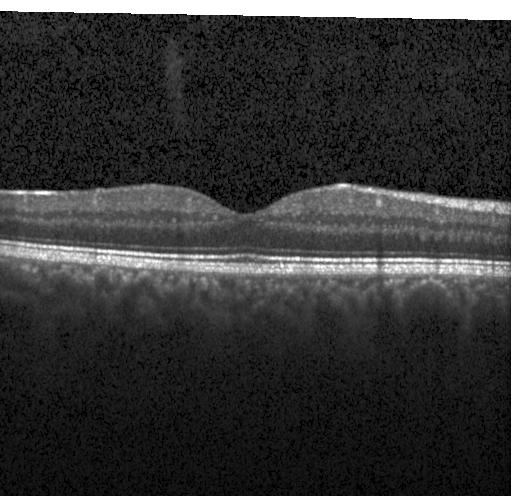

Through the macula; spectral-domain optical coherence tomography; optical coherence tomography B-scan; instrument: Heidelberg Spectralis. Assessment: no choroidal neovascularization, no diabetic macular edema, and no drusen.